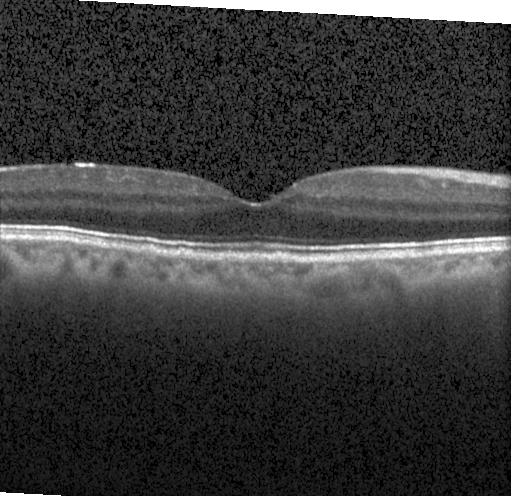

Macular OCT: no CNV, no DME, and no drusen.